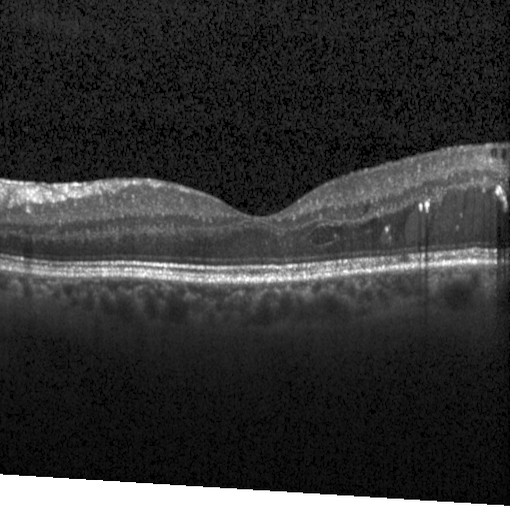

Finding: diabetic macular edema (DME).